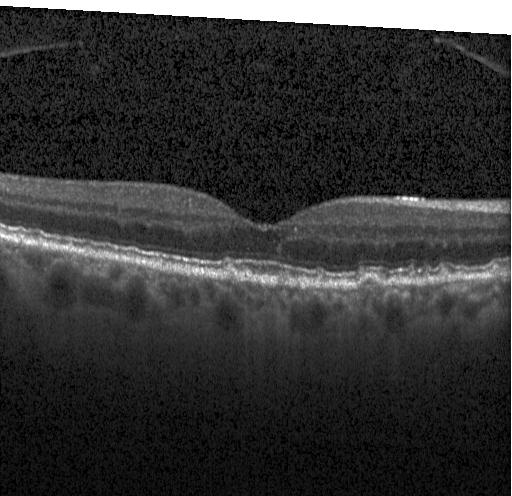
Dx: drusen.